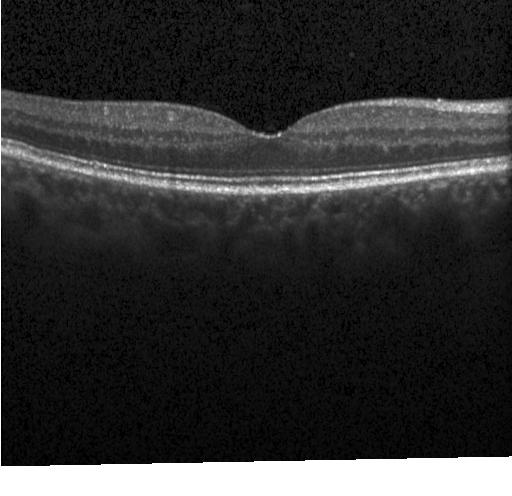
Acquired on a Heidelberg Spectralis, through the macula, spectral-domain optical coherence tomography, retinal OCT cross-section
Diagnosis: no choroidal neovascularization, diabetic macular edema, or drusen.